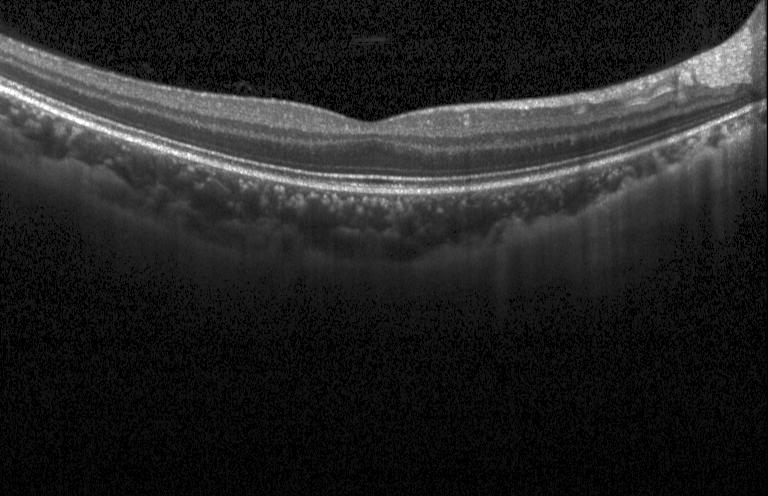
OCT scan showing neither choroidal neovascularization, diabetic macular edema, nor drusen.